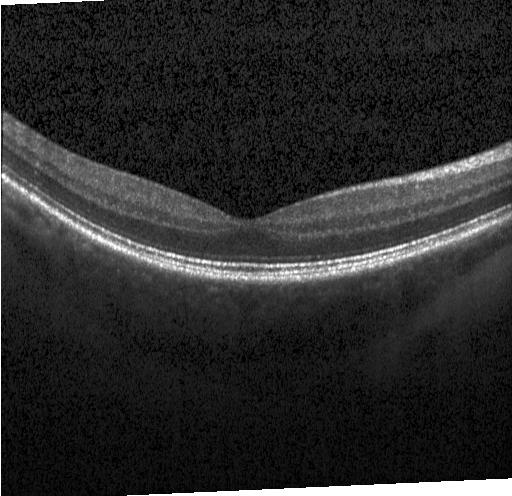

No choroidal neovascularization, no diabetic macular edema, and no drusen.